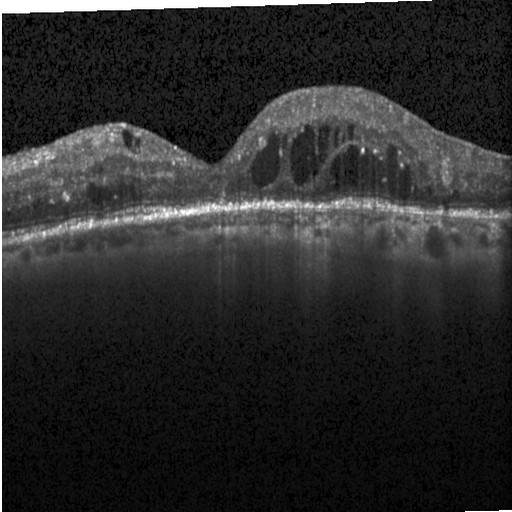 Assessment: diabetic macular edema (DME).